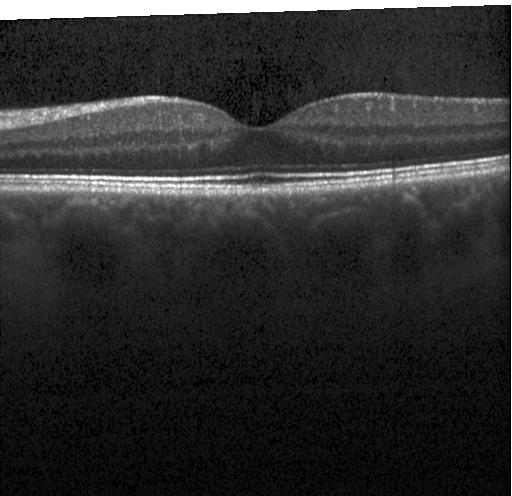 SD-OCT; OCT B-scan; Heidelberg Spectralis OCT system
The scan shows no evidence of choroidal neovascularization, diabetic macular edema, or drusen.